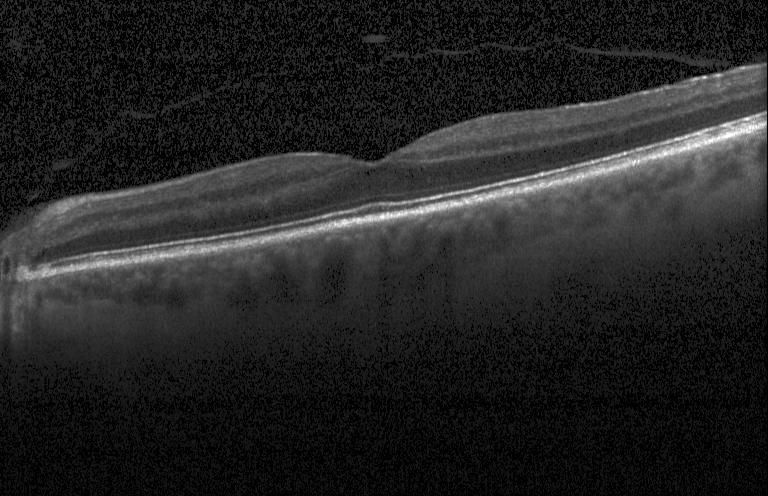
Through the macula · retinal OCT B-scan · acquired on a Heidelberg Spectralis. Impression: no evidence of CNV, DME, or drusen.